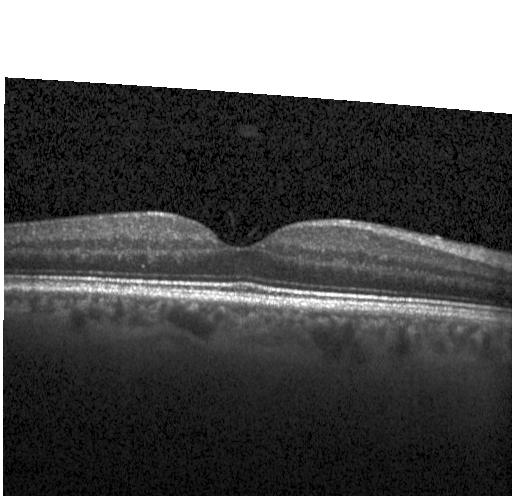

OCT scan showing neither choroidal neovascularization, diabetic macular edema, nor drusen.